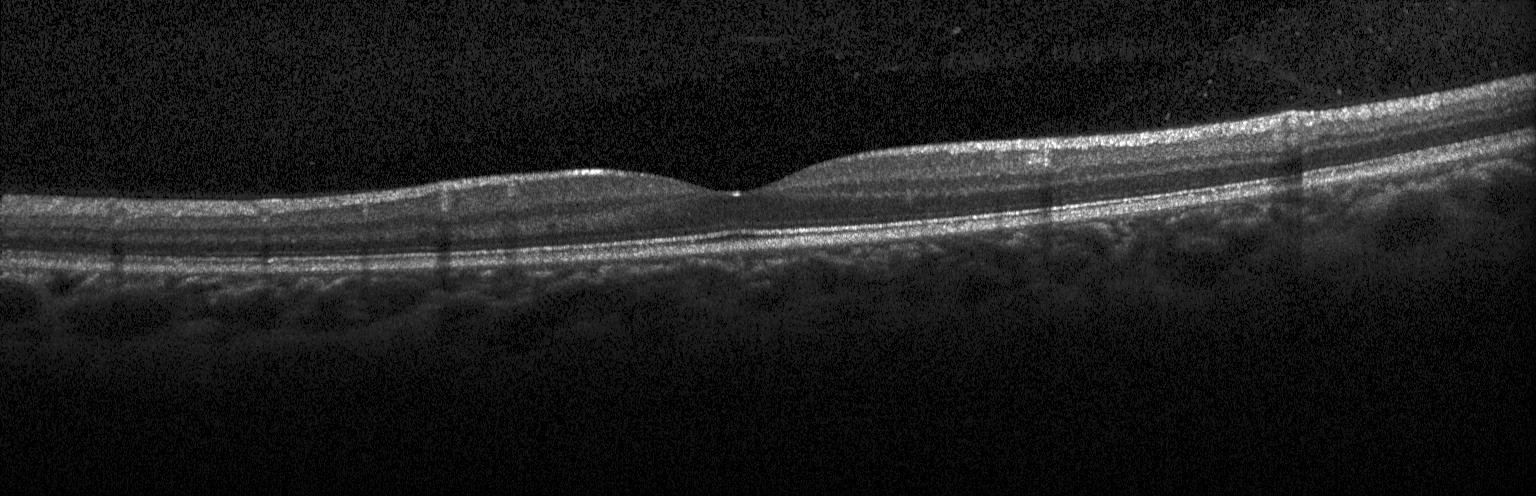

The scan shows neither CNV, DME, nor drusen.